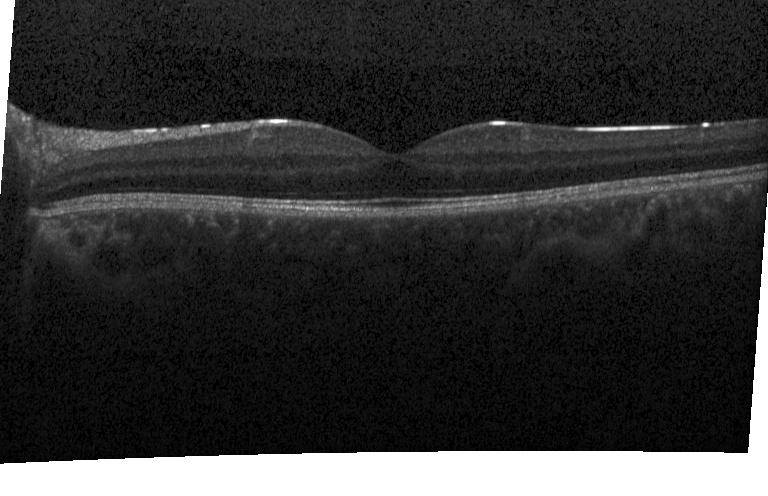 Centered on the fovea. Optical coherence tomography B-scan. Finding: no evidence of CNV, DME, or drusen.